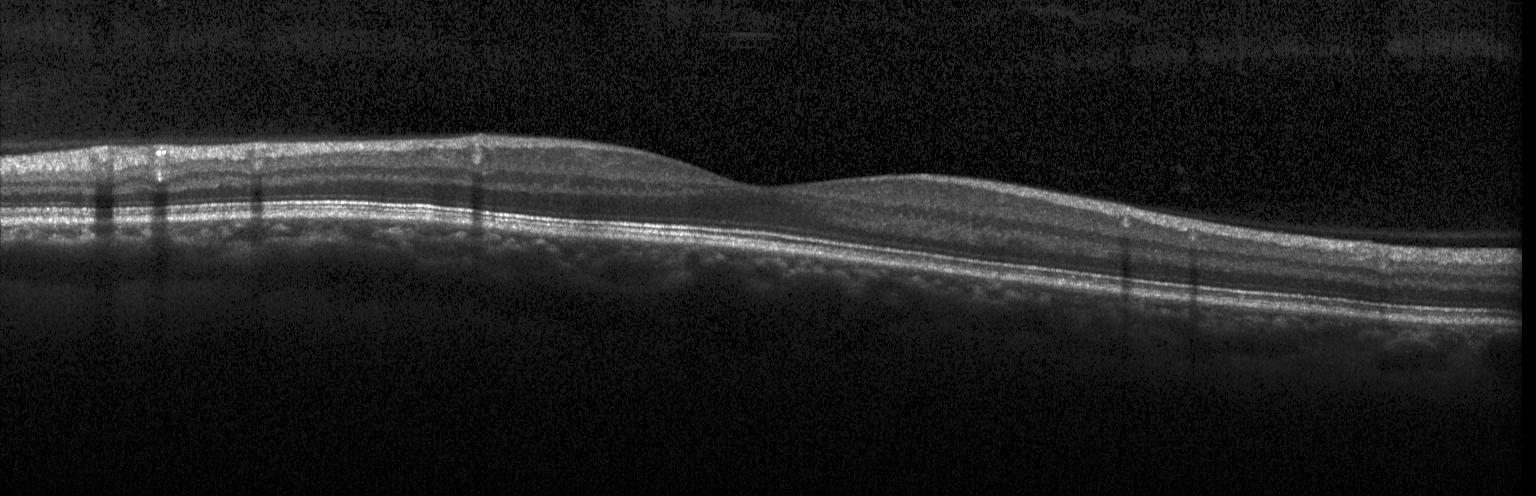 Macular OCT: no evidence of CNV, DME, or drusen.